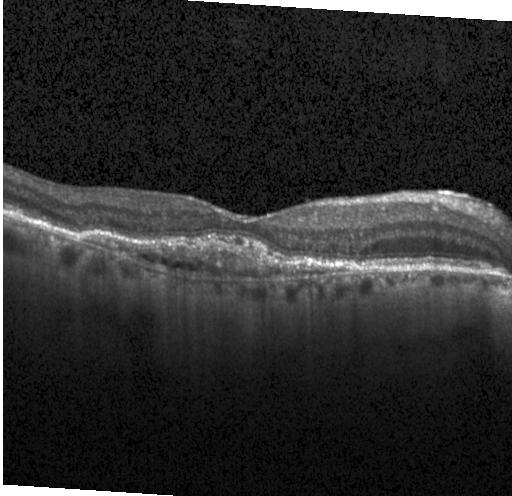

Optical coherence tomography scan; macular scan. Finding: a choroidal neovascular membrane.